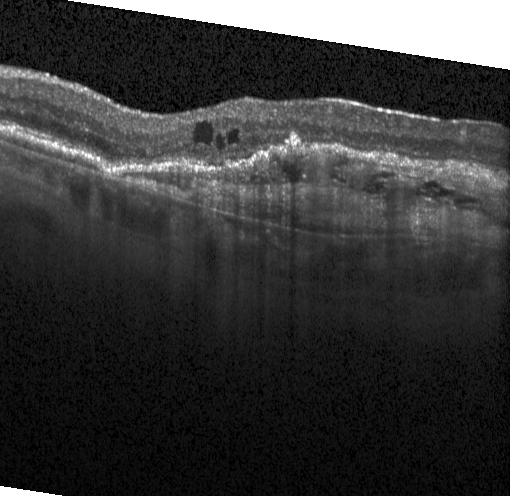
Assessment: CNV.